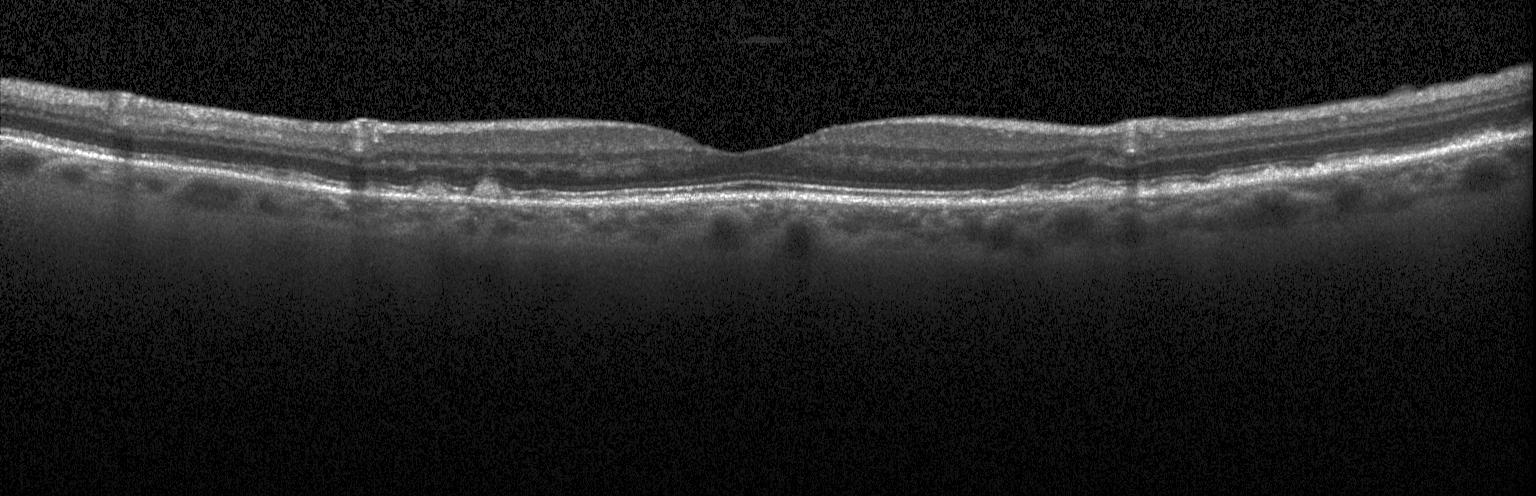 Impression: sub-RPE drusenoid deposits.